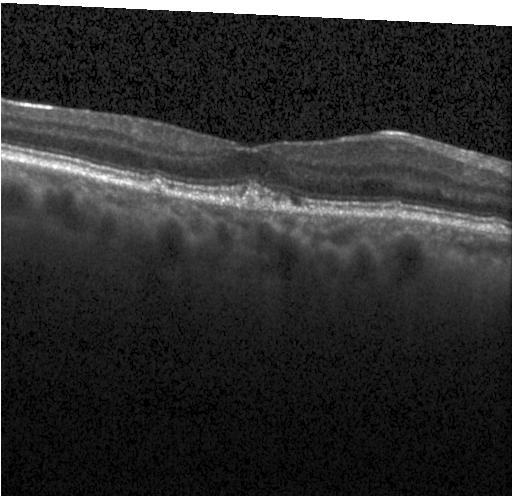
SD-OCT · OCT line scan.
Finding: drusen.